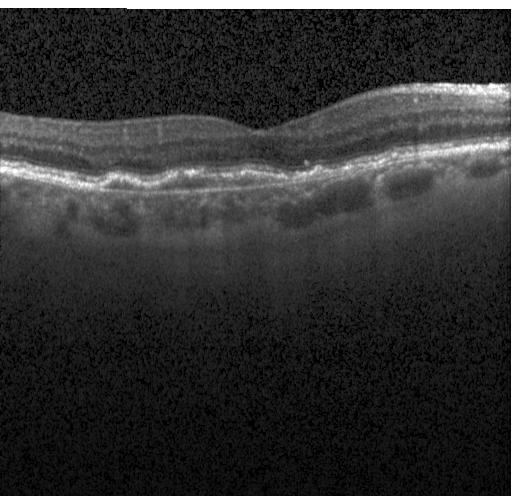

Retinal OCT cross-section. OCT finding: CNV.